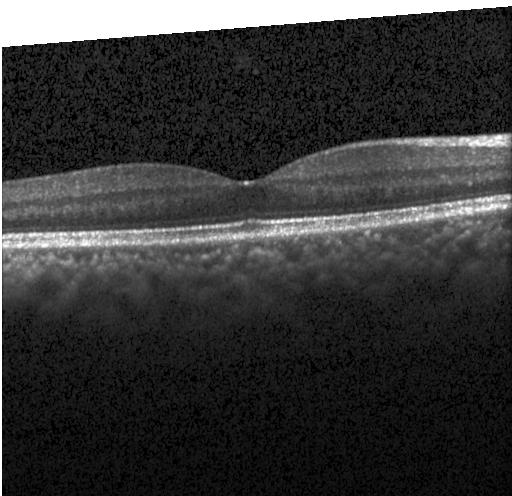

Finding: no evidence of CNV, DME, or drusen.